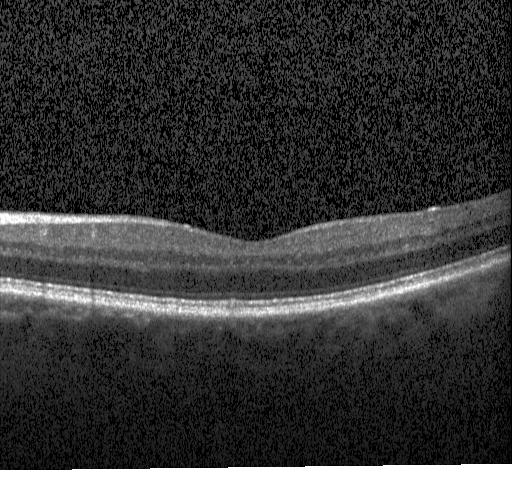 No choroidal neovascularization, diabetic macular edema, or drusen.